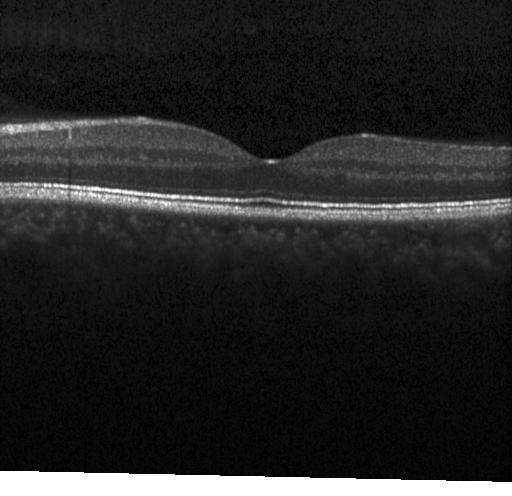
OCT finding: no evidence of choroidal neovascularization, diabetic macular edema, or drusen.